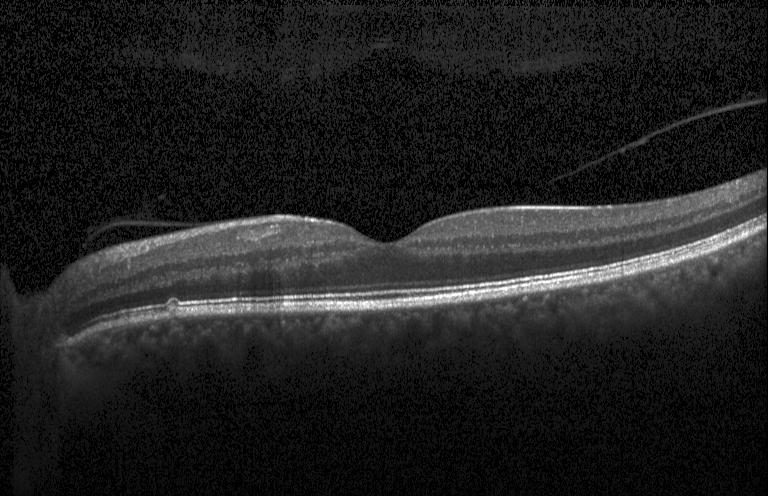
Retinal OCT B-scan, through the macula, spectral-domain OCT, instrument: Heidelberg Spectralis. Assessment: no evidence of choroidal neovascularization, diabetic macular edema, or drusen.